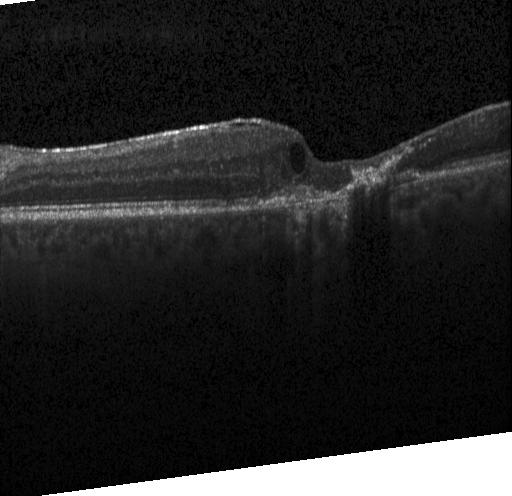
SD-OCT · OCT line scan · acquired on a Heidelberg Spectralis.
Assessment: CNV.